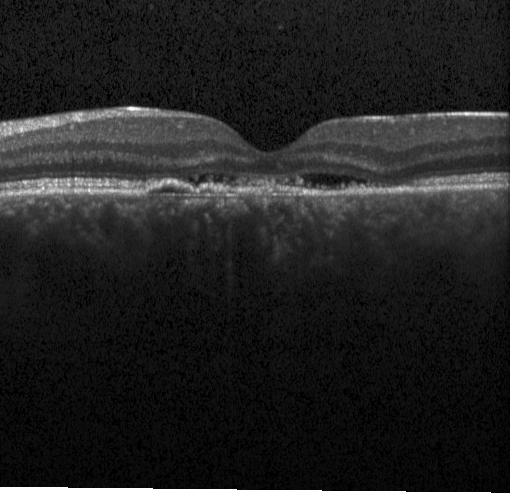 Retinal OCT B-scan; spectral-domain optical coherence tomography; through the macula
Dx: CNV.